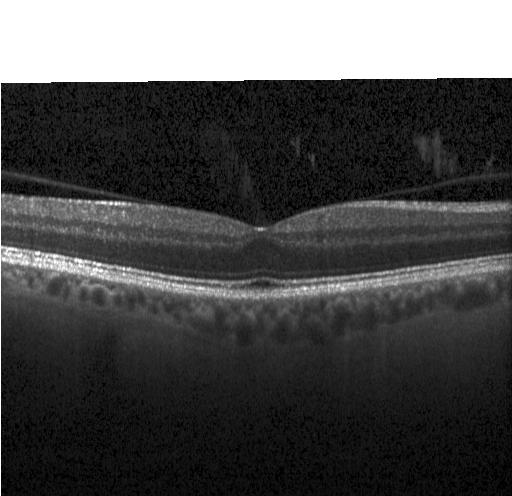

Spectral-domain optical coherence tomography · optical coherence tomography scan · acquired on a Heidelberg Spectralis · fovea-centered
OCT finding: no choroidal neovascularization, no diabetic macular edema, and no drusen.